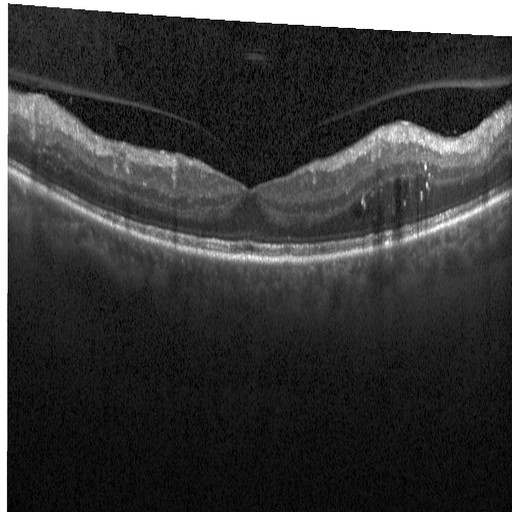

OCT line scan — The scan shows diabetic macular edema.